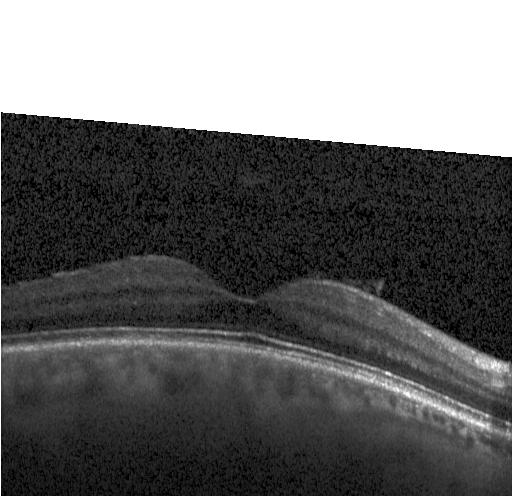 OCT line scan — Diagnosis: no CNV, DME, or drusen.